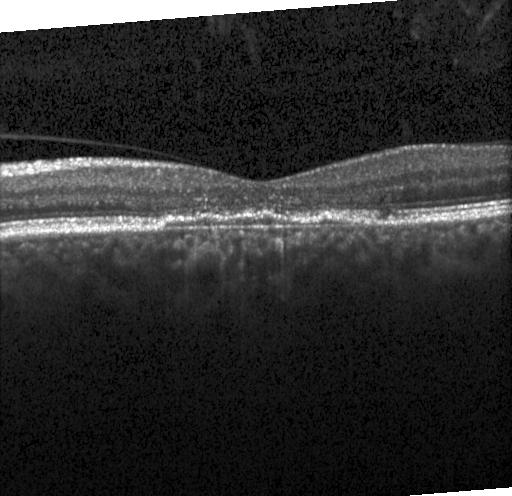

Diagnosis: choroidal neovascularization.